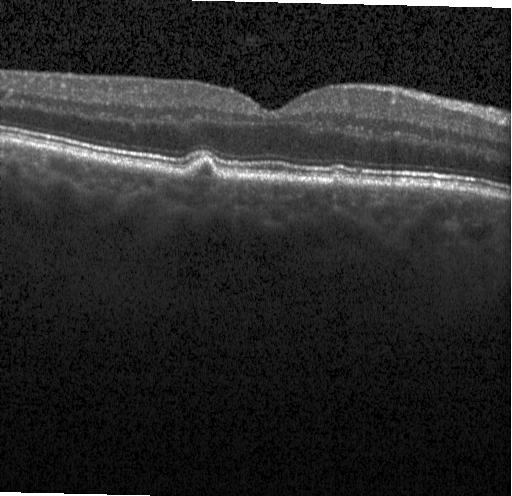

Retinal OCT cross-section. SD-OCT. Instrument: Heidelberg Spectralis. Drusen.